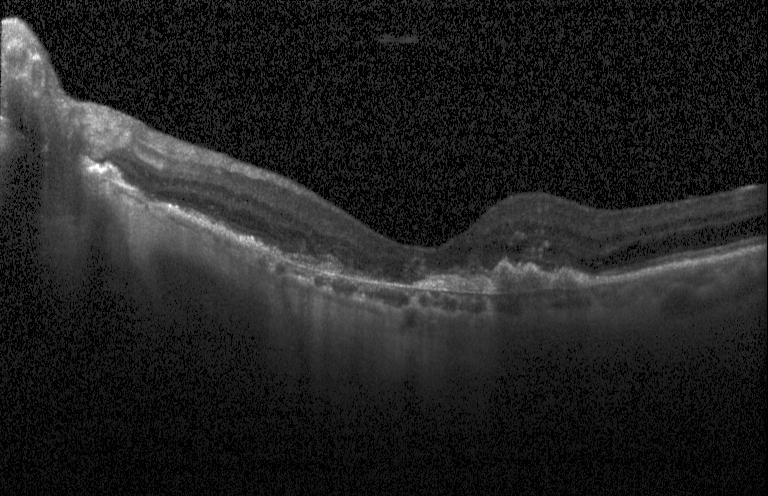 Heidelberg Spectralis OCT system. Optical coherence tomography scan — Impression: a choroidal neovascular membrane.